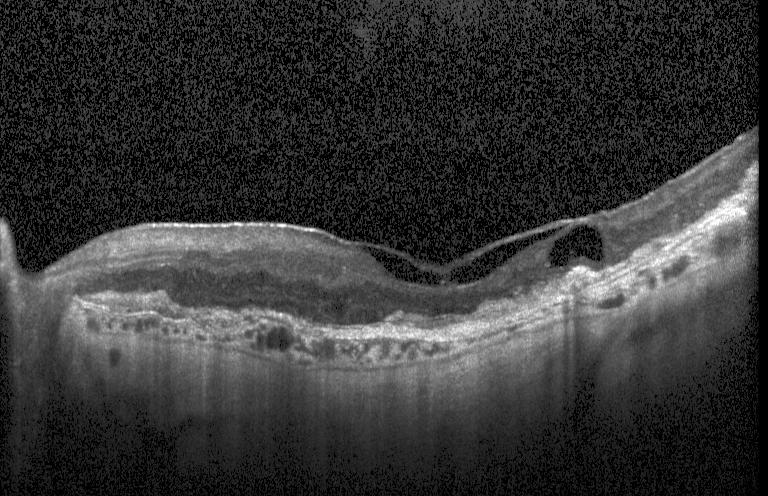
SD-OCT · retinal OCT B-scan. Dx: choroidal neovascularization (CNV).